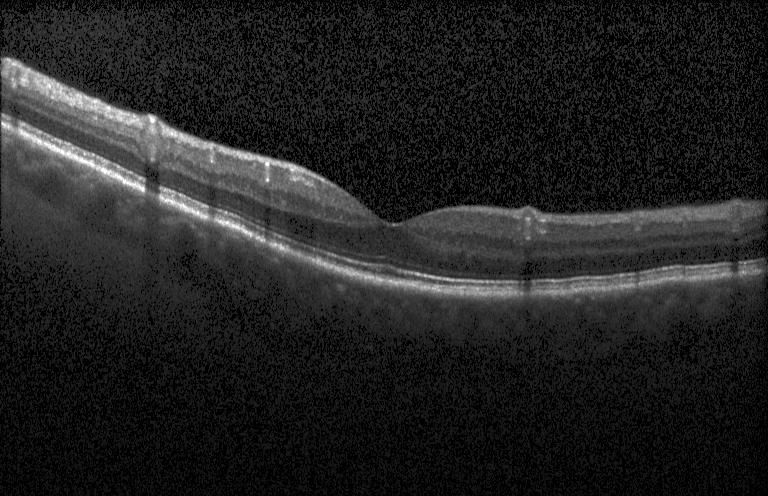 Macular scan · spectral-domain optical coherence tomography · OCT line scan
Diagnosis: no CNV, no DME, and no drusen.